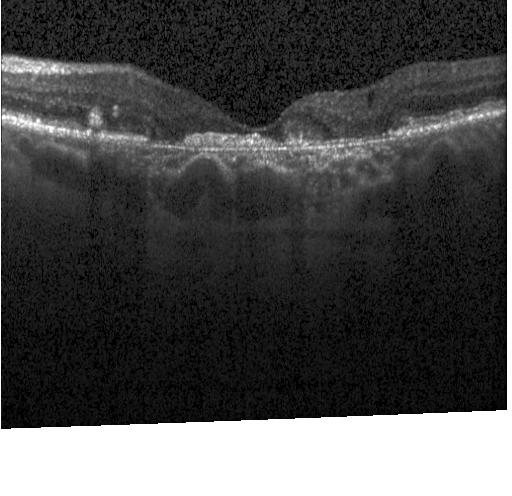
Spectral-domain OCT B-scan: a choroidal neovascular membrane.